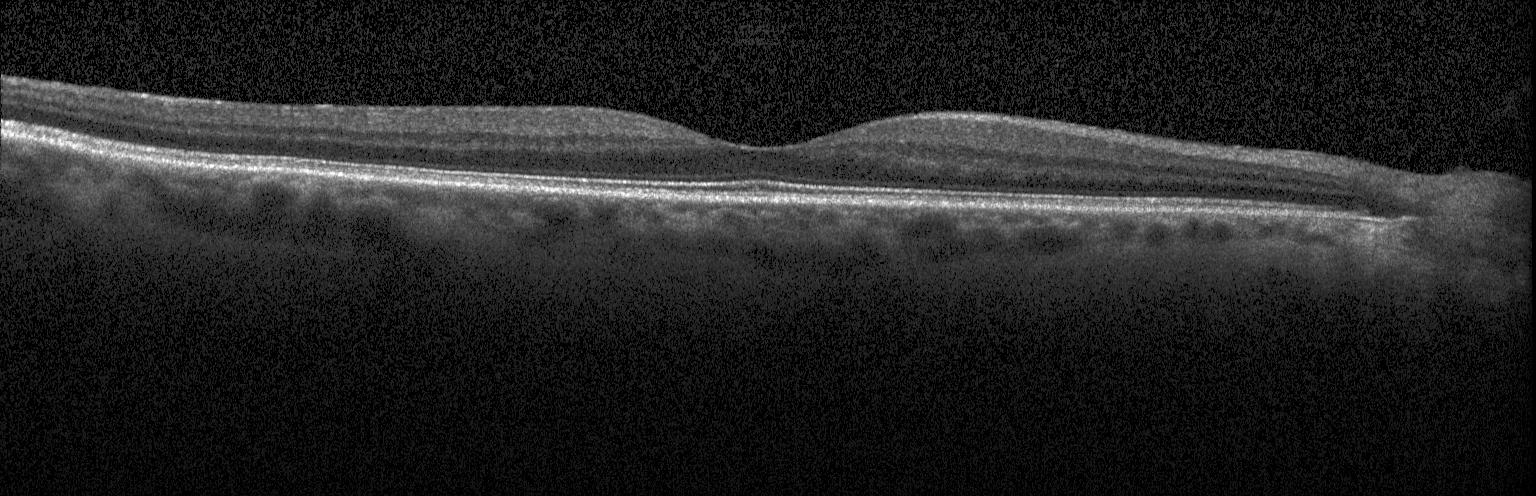
Retinal OCT cross-section · Heidelberg Spectralis OCT system
OCT finding: no choroidal neovascularization, diabetic macular edema, or drusen.